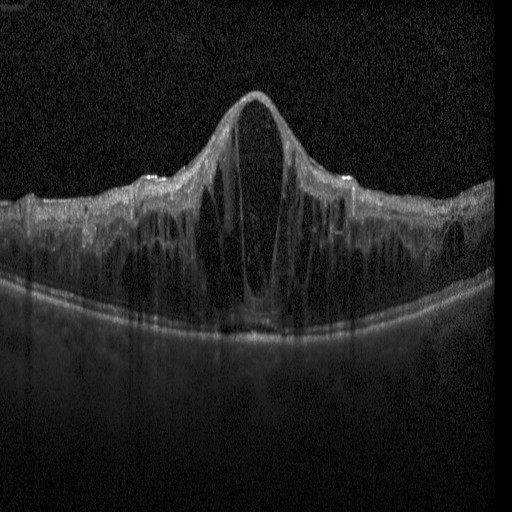 Retinal OCT B-scan · horizontal scan through the fovea
Diagnosis: diabetic macular edema.